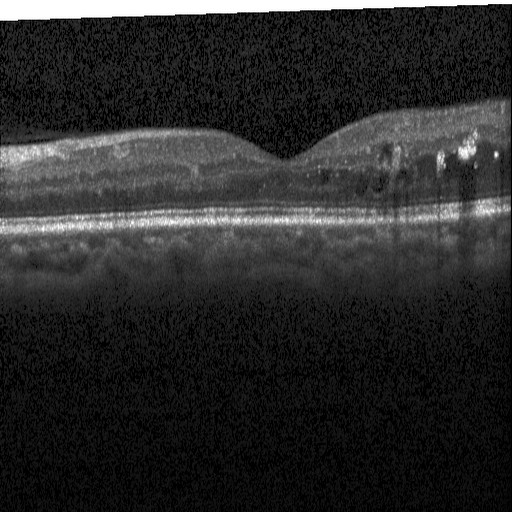 Instrument: Heidelberg Spectralis · OCT B-scan · spectral-domain OCT · horizontal scan through the fovea.
Impression: diabetic macular edema.